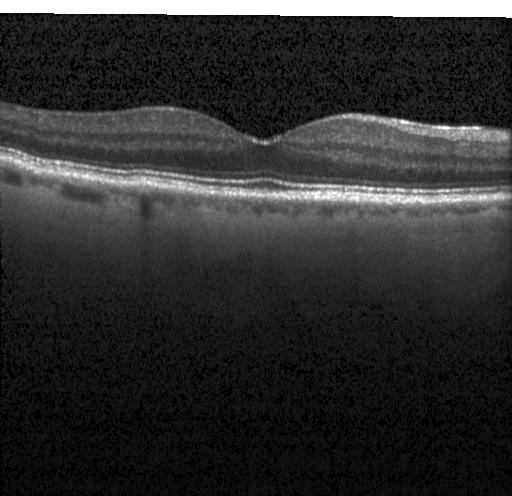

Impression: neither CNV, DME, nor drusen.